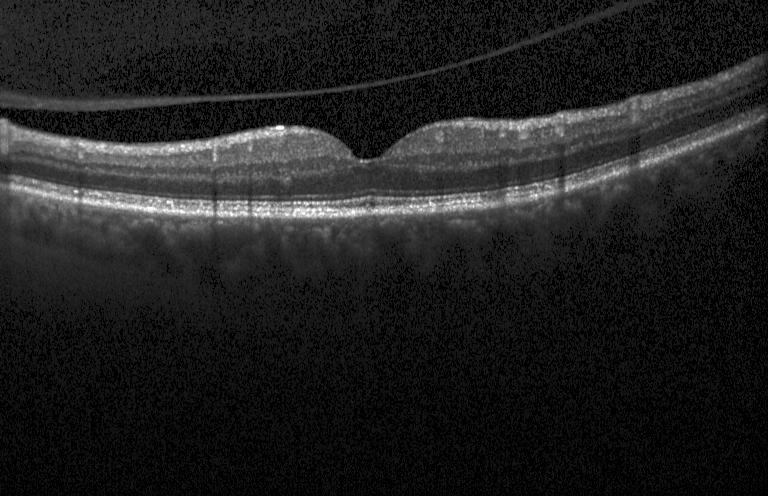

OCT B-scan
Macular OCT: no choroidal neovascularization, diabetic macular edema, or drusen.